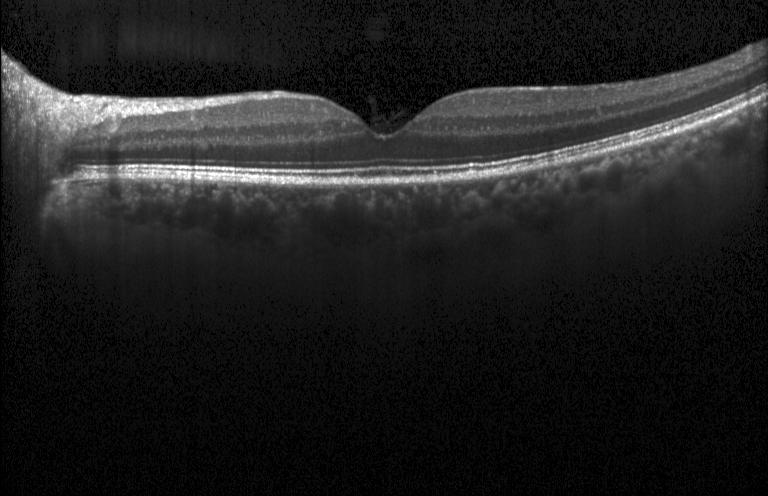

Retinal OCT cross-section. SD-OCT. Macular scan
The scan shows no choroidal neovascularization, no diabetic macular edema, and no drusen.